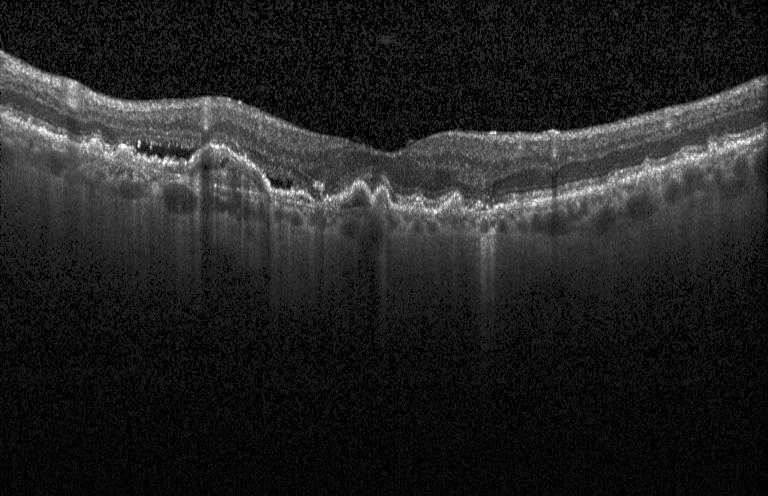 Retinal OCT cross-section · macular scan · spectral-domain optical coherence tomography. A choroidal neovascular membrane.